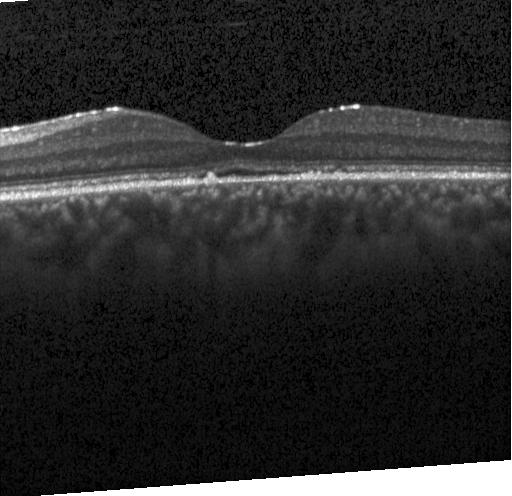 Horizontal scan through the fovea. Spectral-domain OCT. OCT B-scan.
No CNV, DME, or drusen.